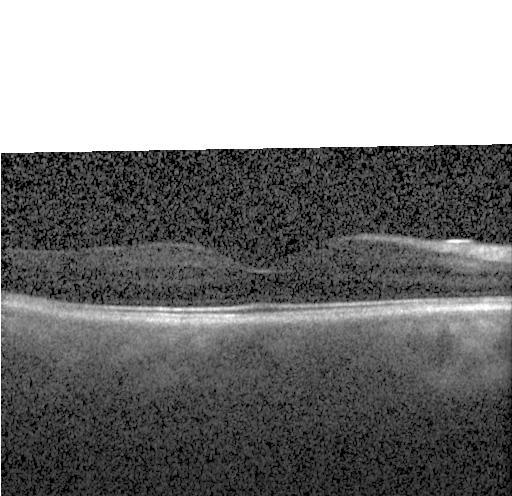

Heidelberg Spectralis. Optical coherence tomography B-scan.
OCT finding: no CNV, no DME, and no drusen.